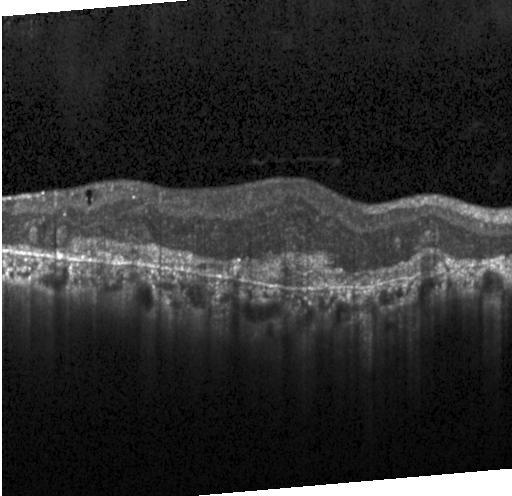

Optical coherence tomography scan · spectral-domain optical coherence tomography · centered on the fovea — Diagnosis: CNV.